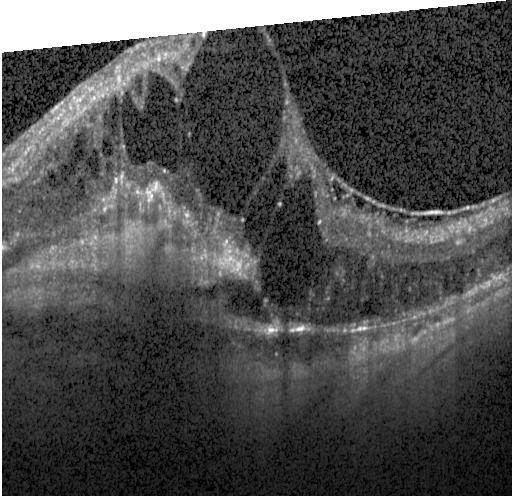
The scan shows a choroidal neovascular membrane.